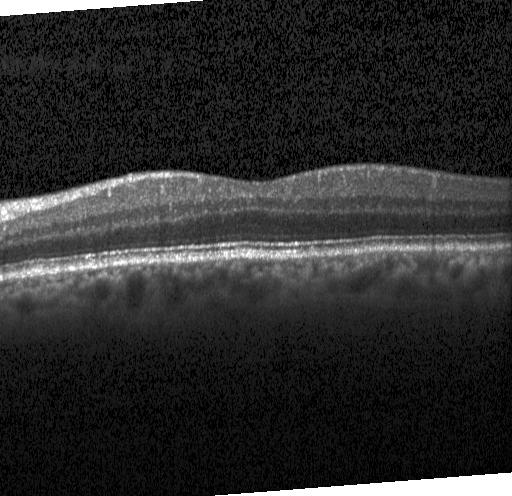

Spectral-domain OCT B-scan: no evidence of choroidal neovascularization, diabetic macular edema, or drusen.